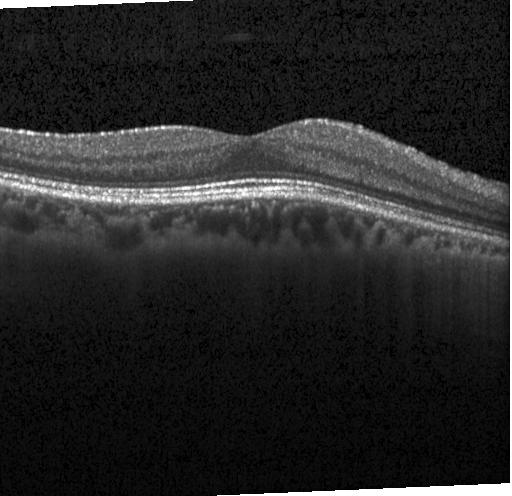

Spectral-domain optical coherence tomography; OCT line scan. Diagnosis: no choroidal neovascularization, no diabetic macular edema, and no drusen.